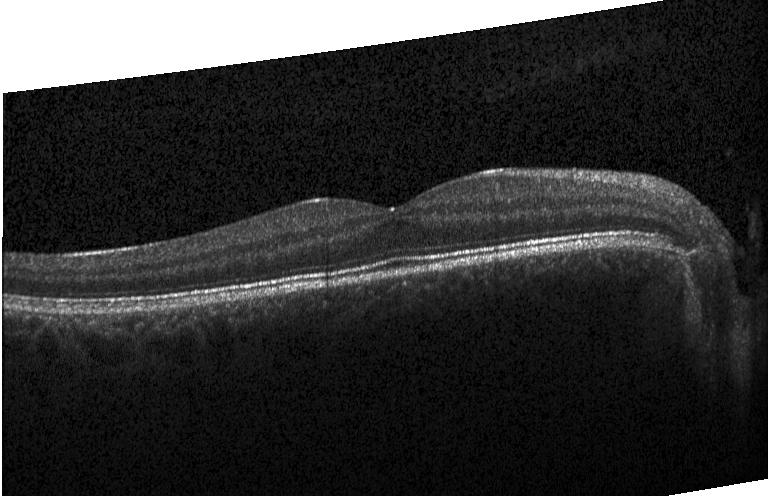 OCT line scan — Assessment: no evidence of choroidal neovascularization, diabetic macular edema, or drusen.